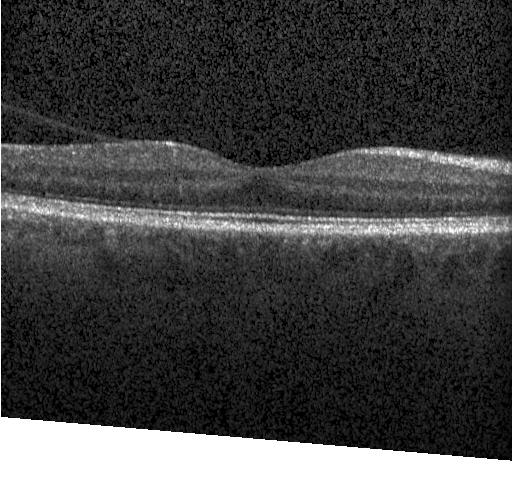

Instrument: Heidelberg Spectralis, optical coherence tomography B-scan — Diagnosis: neither choroidal neovascularization, diabetic macular edema, nor drusen.